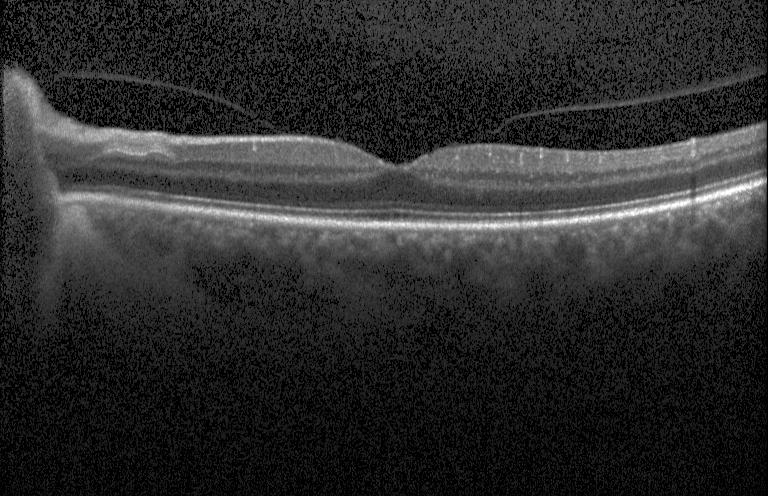

Spectral-domain OCT, OCT B-scan, acquired on a Heidelberg Spectralis, macular scan — Finding: no choroidal neovascularization, no diabetic macular edema, and no drusen.